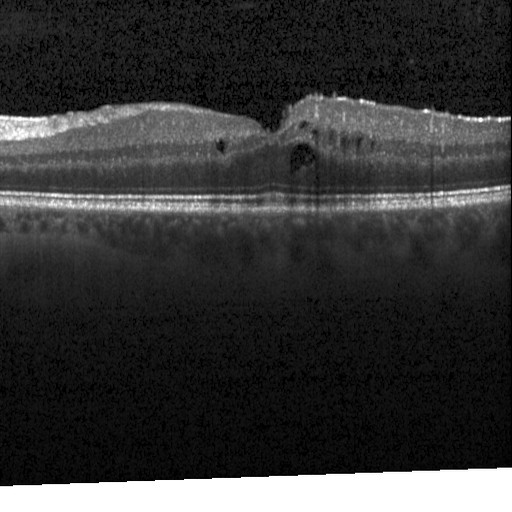

Optical coherence tomography scan, horizontal scan through the fovea
Diagnosis: DME.